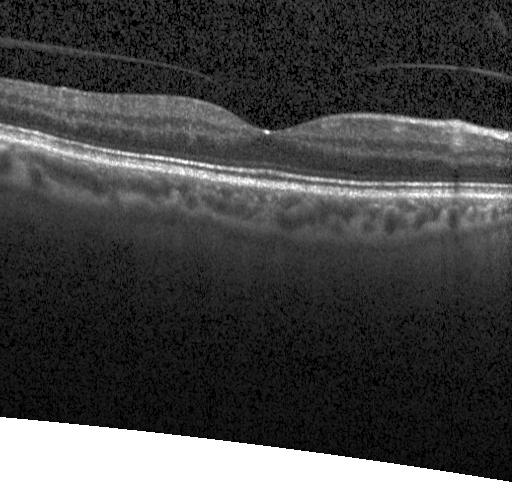
Retinal OCT cross-section showing no choroidal neovascularization, diabetic macular edema, or drusen.